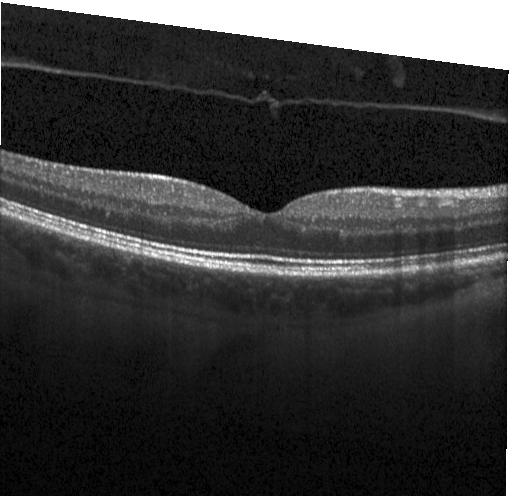
Dx: neither choroidal neovascularization, diabetic macular edema, nor drusen.